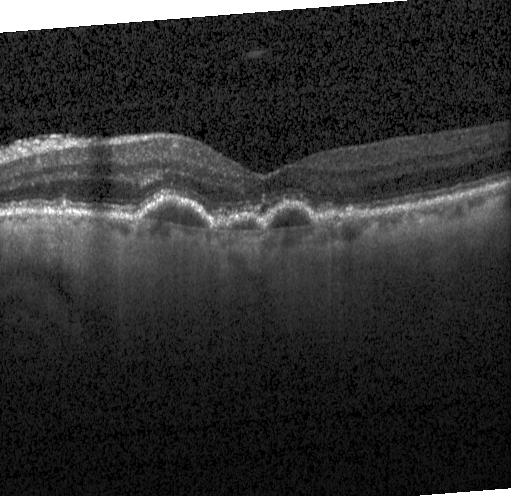
Heidelberg Spectralis; centered on the fovea; SD-OCT; optical coherence tomography B-scan. Impression: CNV.